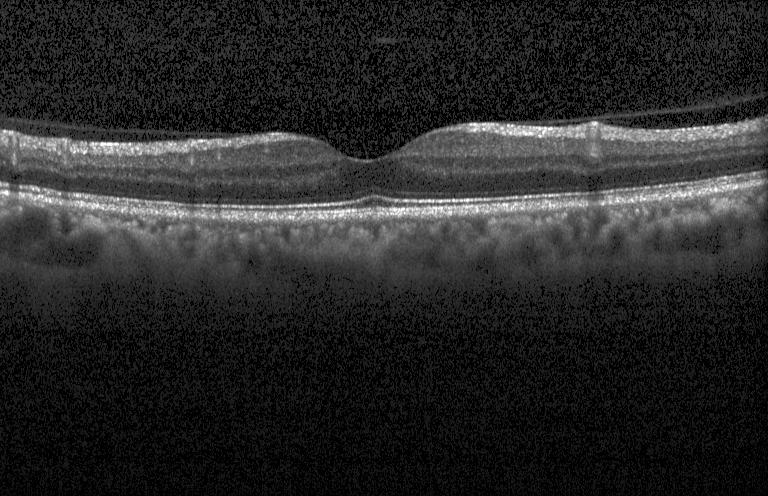
Retinal OCT cross-section
This B-scan demonstrates no choroidal neovascularization, diabetic macular edema, or drusen.